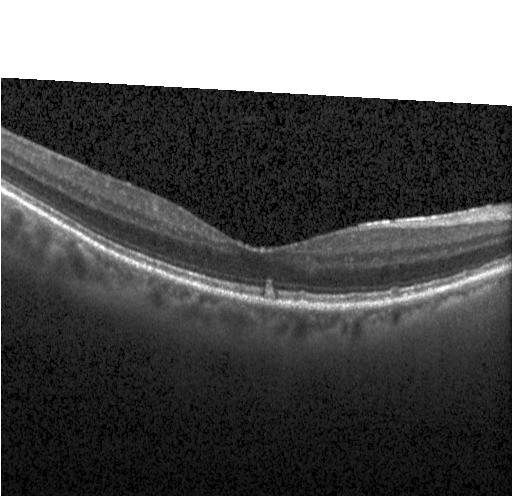 Macular OCT: sub-RPE drusenoid deposits.